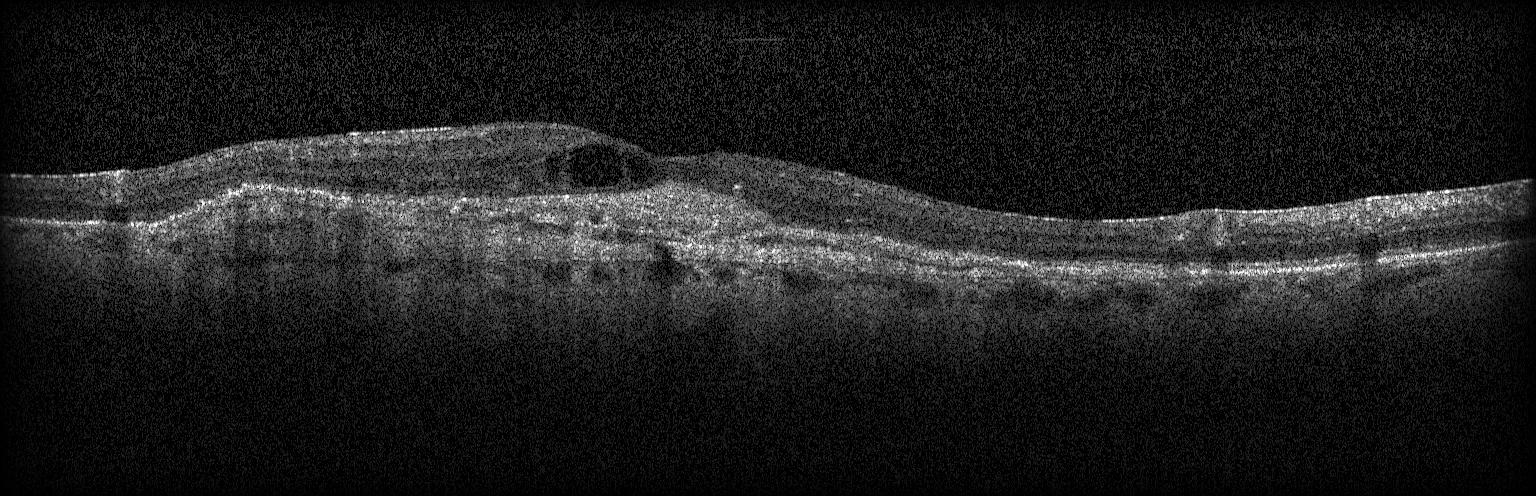
This B-scan demonstrates choroidal neovascularization.